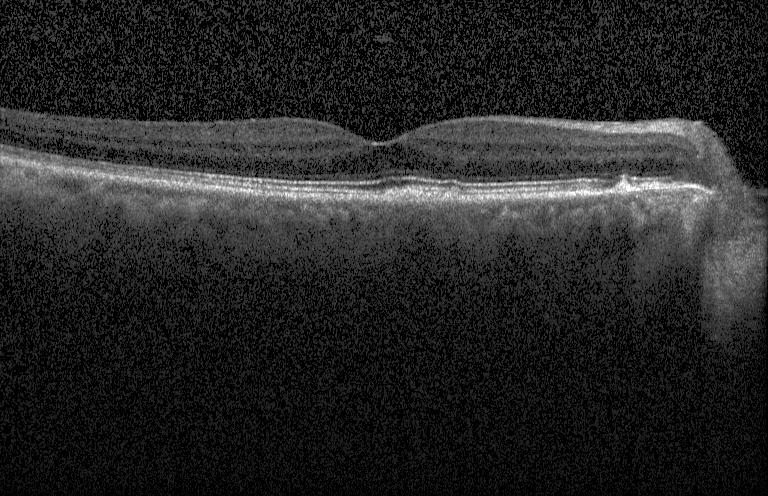
Optical coherence tomography scan · spectral-domain OCT · through the macula — This B-scan demonstrates drusen.